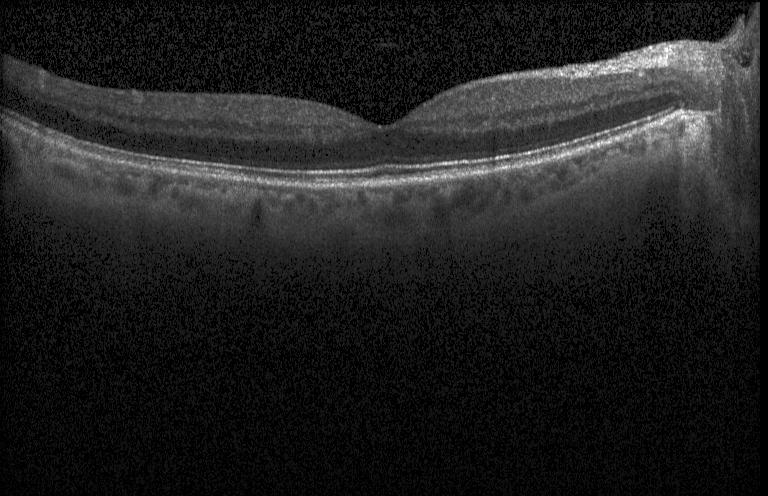 OCT finding: neither choroidal neovascularization, diabetic macular edema, nor drusen.